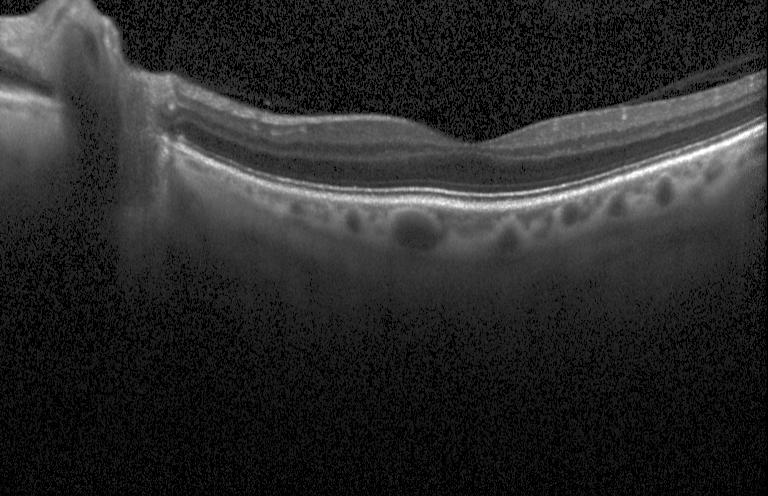
Through the macula; Heidelberg Spectralis; optical coherence tomography scan; SD-OCT.
Impression: no evidence of choroidal neovascularization, diabetic macular edema, or drusen.